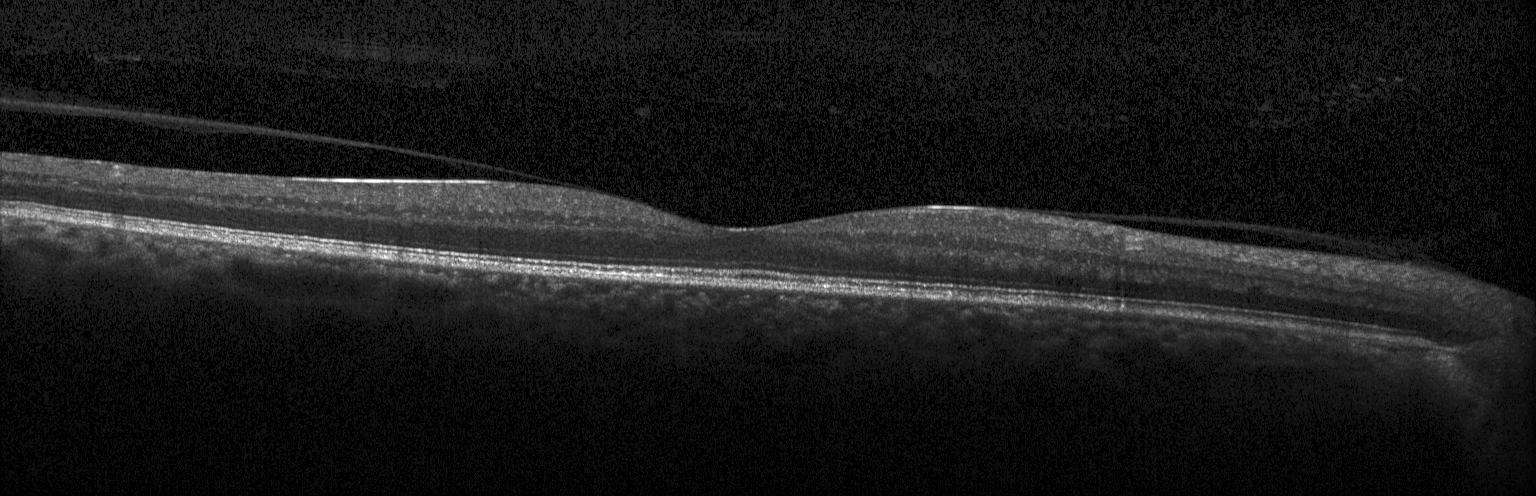
Assessment: neither choroidal neovascularization, diabetic macular edema, nor drusen.